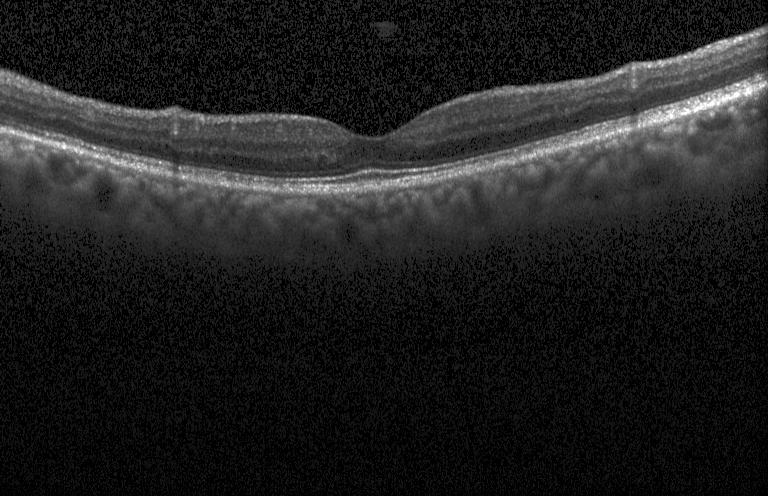 The scan shows neither choroidal neovascularization, diabetic macular edema, nor drusen.